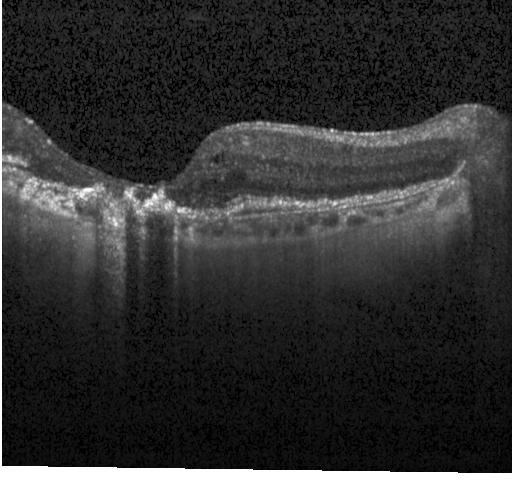
Retinal OCT B-scan — Diagnosis: a choroidal neovascular membrane.